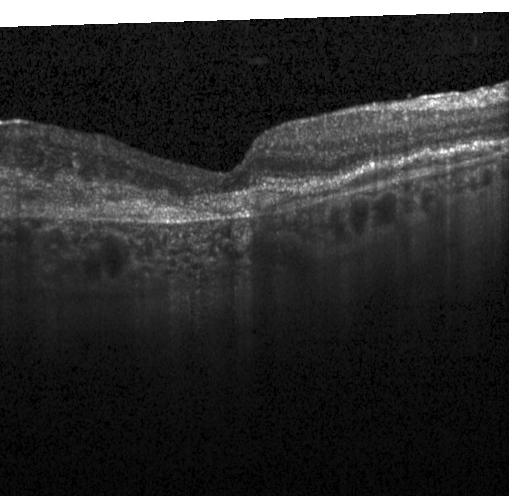
OCT B-scan; macular scan; Heidelberg Spectralis OCT system — Finding: a choroidal neovascular membrane.